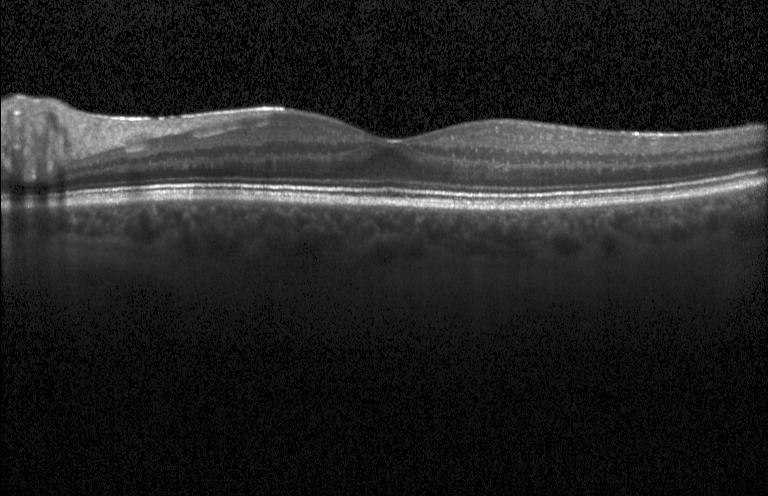 Diagnosis: neither choroidal neovascularization, diabetic macular edema, nor drusen.